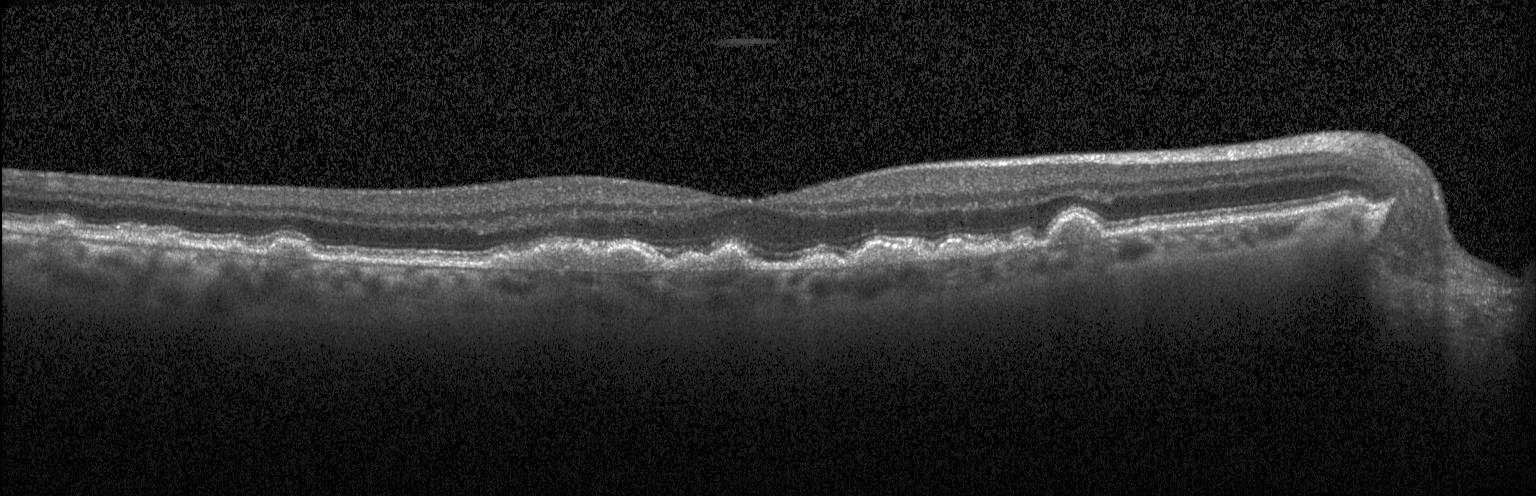

Macular scan · optical coherence tomography scan · Heidelberg Spectralis OCT system · spectral-domain OCT. Assessment: sub-RPE drusenoid deposits.